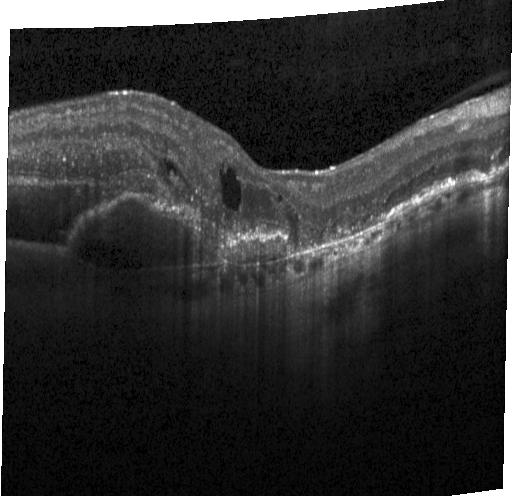

OCT B-scan
Finding: CNV.